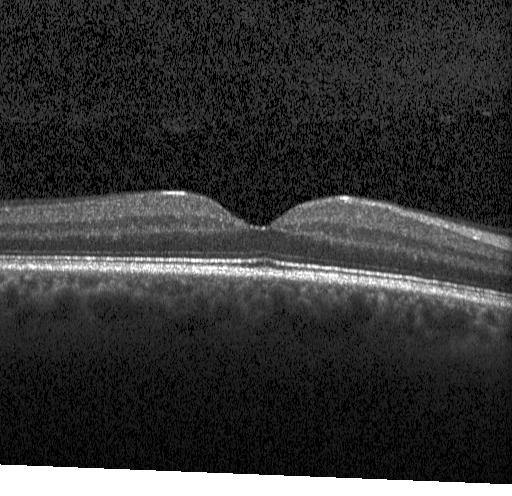 Dx: no choroidal neovascularization, no diabetic macular edema, and no drusen.